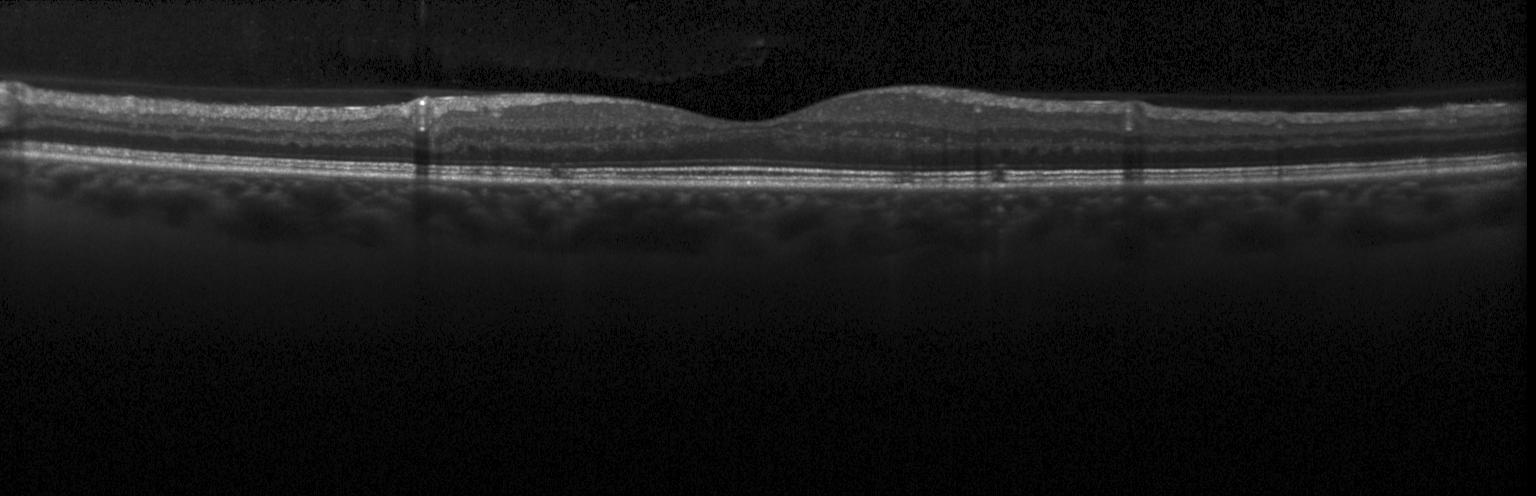
Impression: no choroidal neovascularization, no diabetic macular edema, and no drusen.